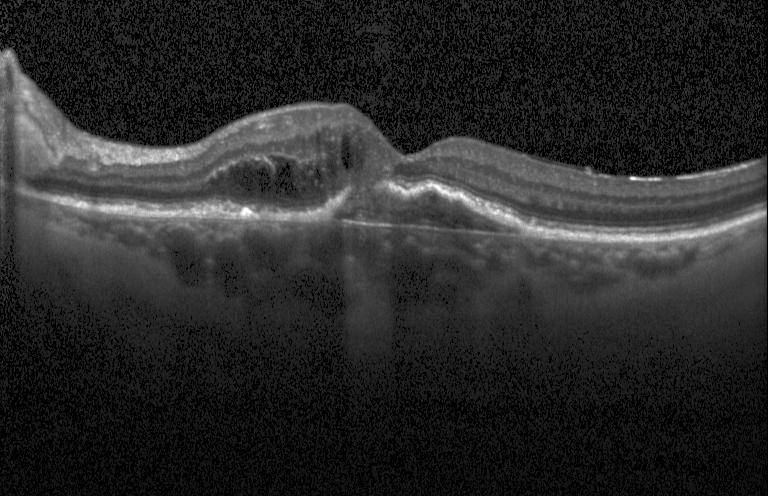
OCT scan showing a choroidal neovascular membrane.